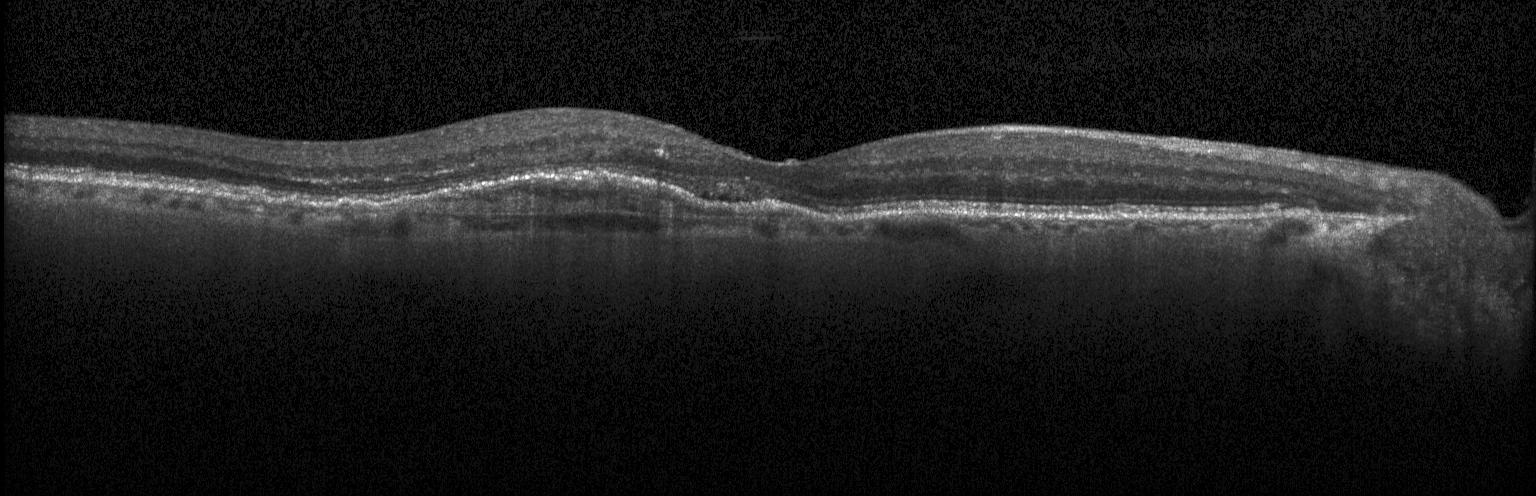 Impression: a choroidal neovascular membrane.